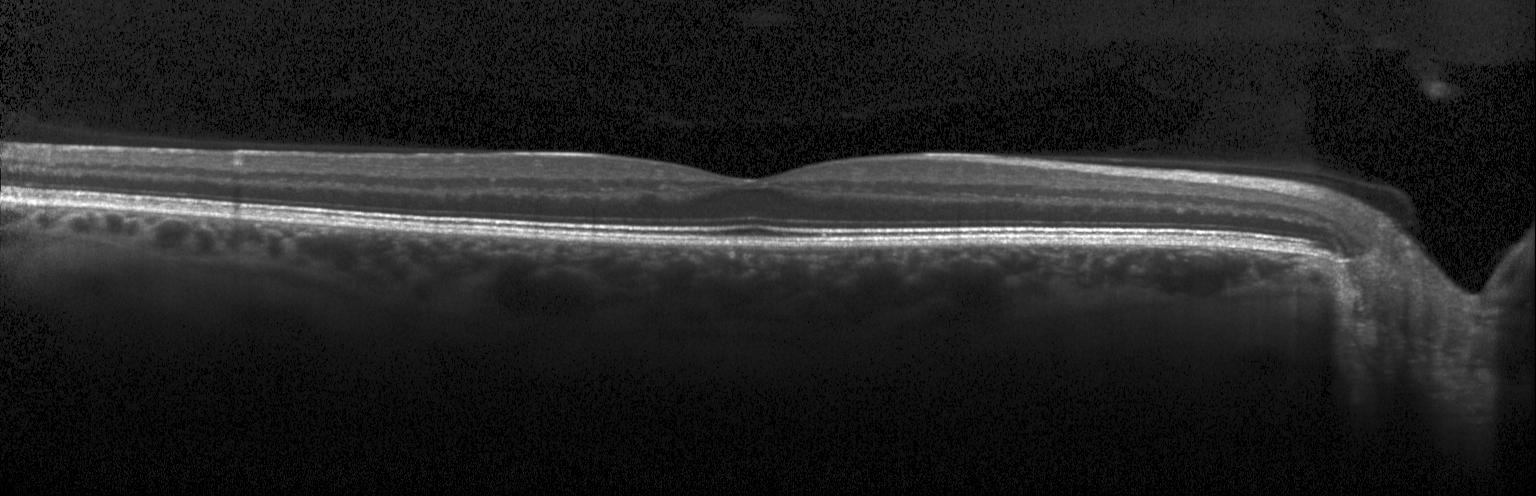

Heidelberg Spectralis OCT system · spectral-domain optical coherence tomography · horizontal scan through the fovea · optical coherence tomography B-scan.
Diagnosis: no choroidal neovascularization, diabetic macular edema, or drusen.